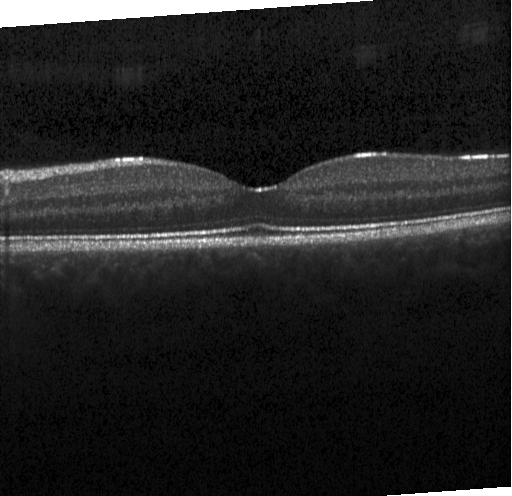 OCT line scan, macular scan, SD-OCT, instrument: Heidelberg Spectralis. Dx: no CNV, DME, or drusen.